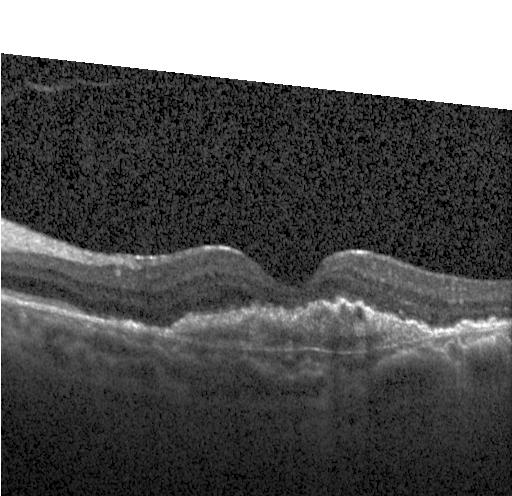
Spectral-domain OCT; macular scan; optical coherence tomography B-scan. This B-scan demonstrates a choroidal neovascular membrane.